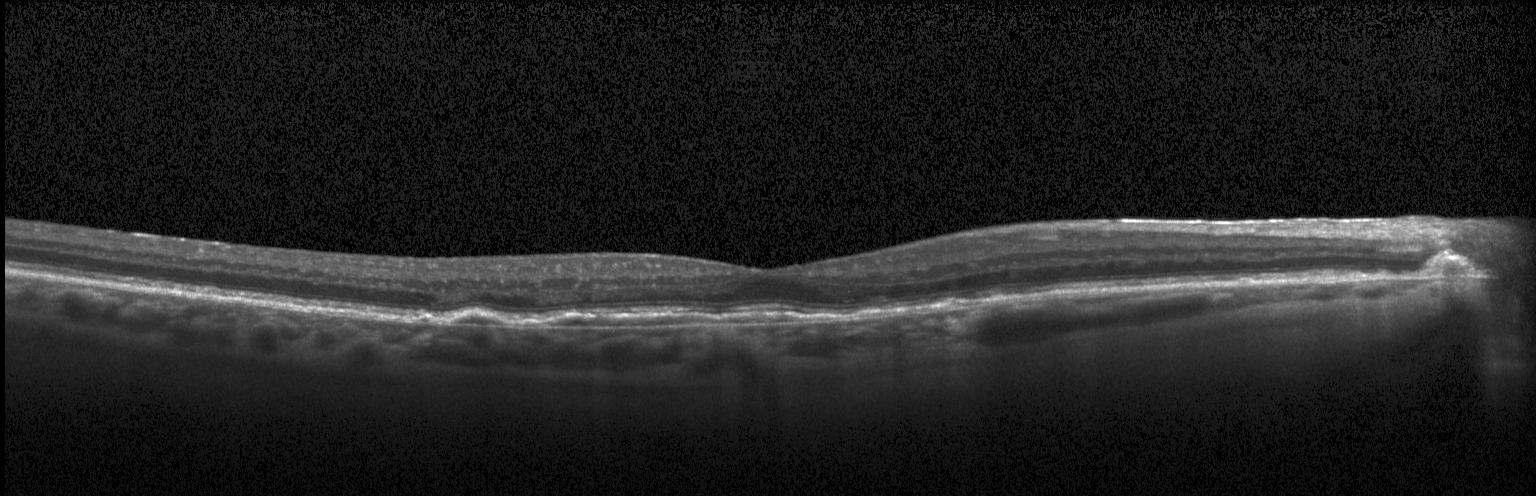 Acquired on a Heidelberg Spectralis. Spectral-domain OCT. OCT B-scan. A choroidal neovascular membrane.